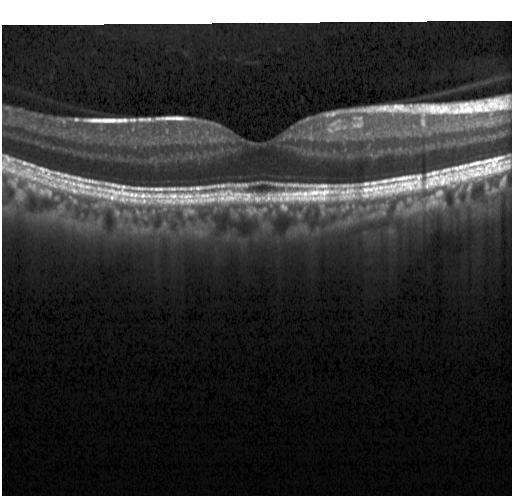 OCT B-scan showing neither choroidal neovascularization, diabetic macular edema, nor drusen.